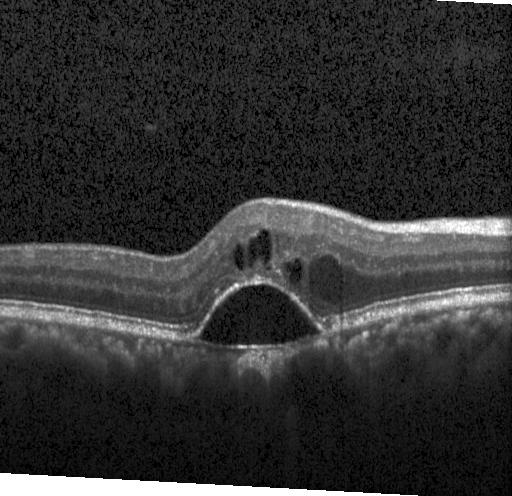
Spectral-domain optical coherence tomography, Heidelberg Spectralis OCT system, retinal OCT cross-section
Macular OCT: CNV.